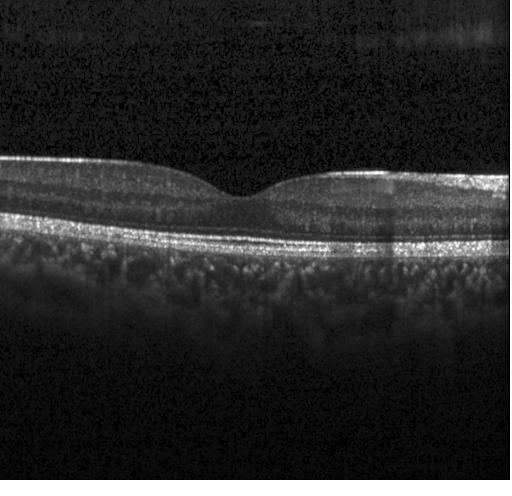 Spectral-domain OCT; horizontal scan through the fovea; retinal OCT cross-section. Diagnosis: no evidence of CNV, DME, or drusen.